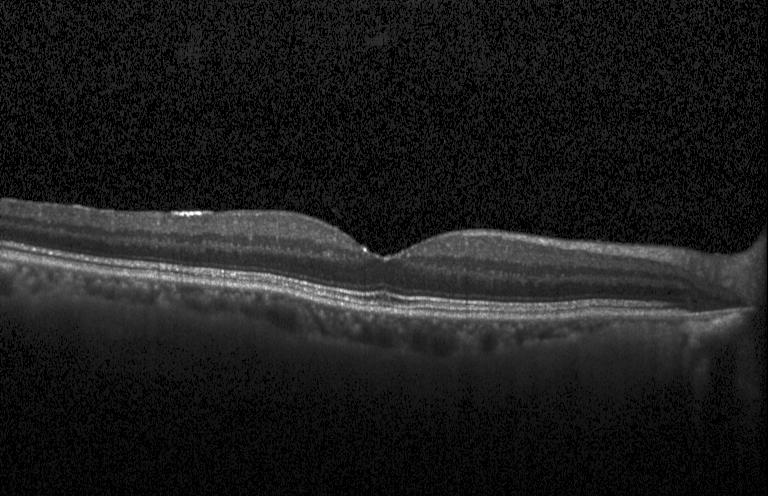 Centered on the fovea, retinal OCT B-scan, SD-OCT — Macular OCT: neither choroidal neovascularization, diabetic macular edema, nor drusen.